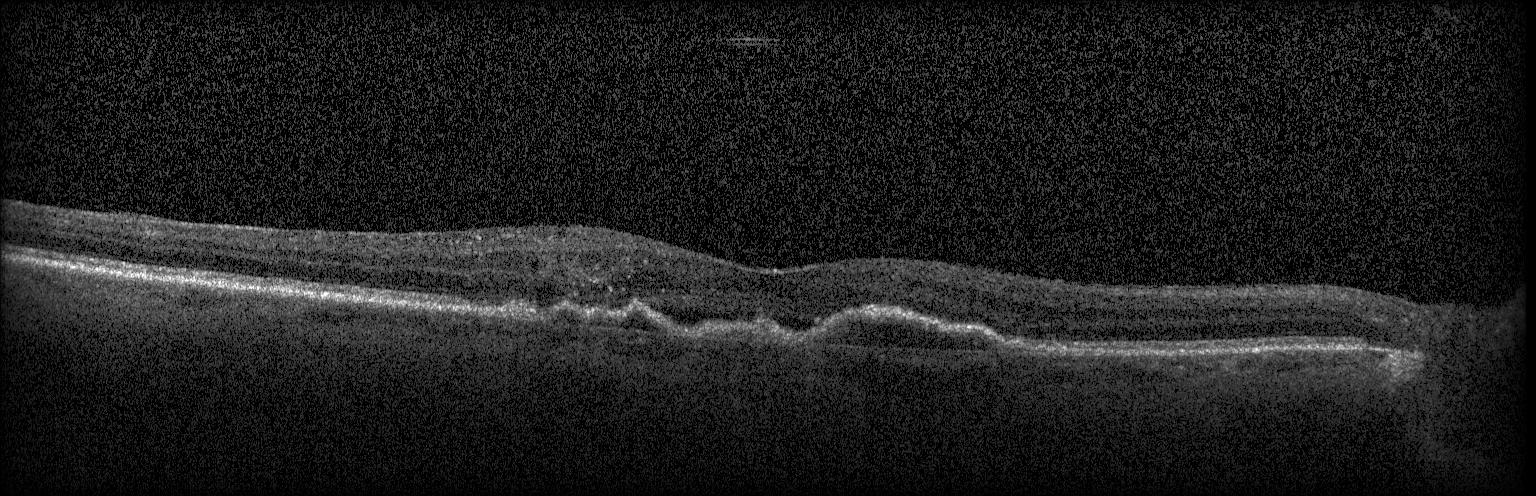 Finding: CNV.